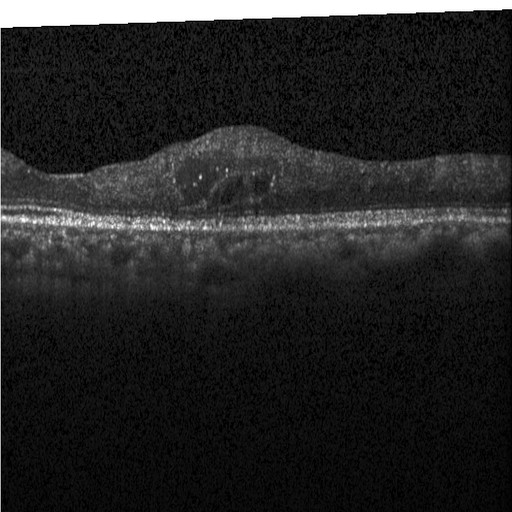

OCT B-scan — Assessment: DME.